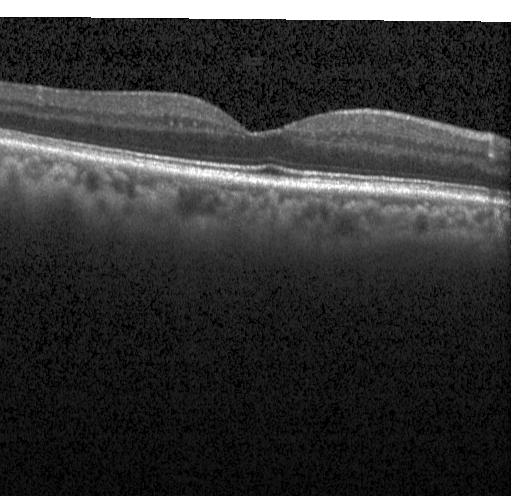

Retinal OCT cross-section.
Impression: no evidence of CNV, DME, or drusen.